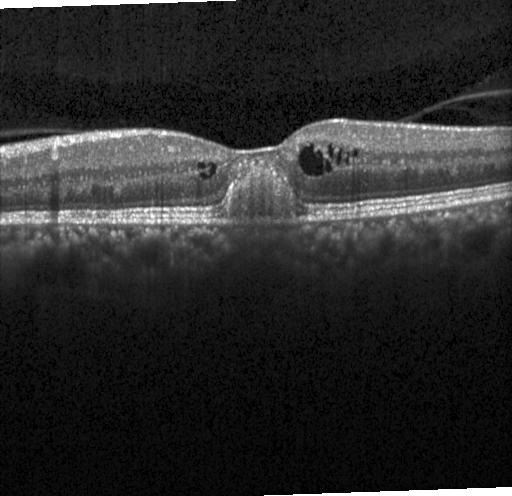 OCT scan showing choroidal neovascularization (CNV).